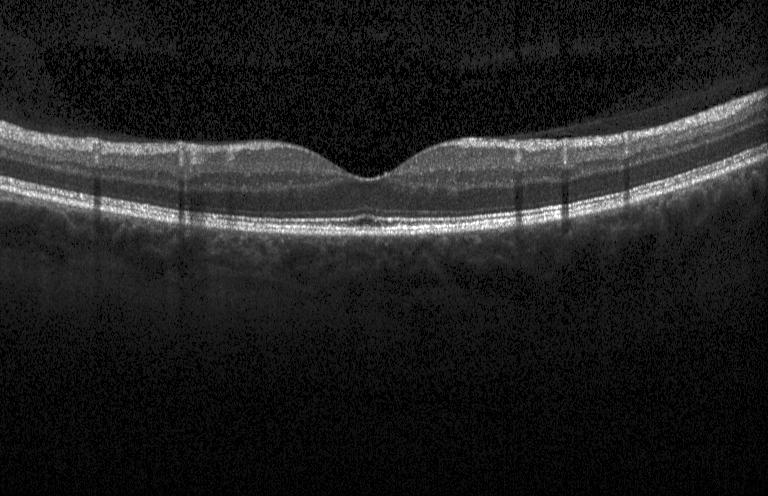
Diagnosis: neither choroidal neovascularization, diabetic macular edema, nor drusen.